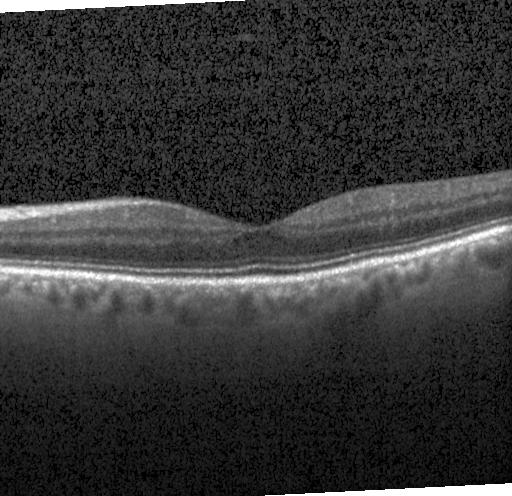 Optical coherence tomography B-scan
Macular OCT: no choroidal neovascularization, diabetic macular edema, or drusen.